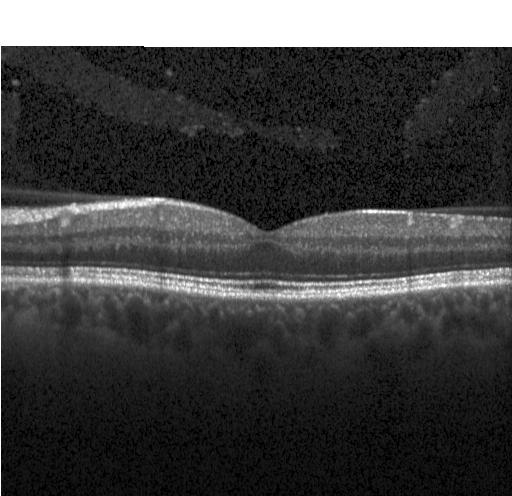 Retinal OCT cross-section.
Macular OCT: no choroidal neovascularization, no diabetic macular edema, and no drusen.